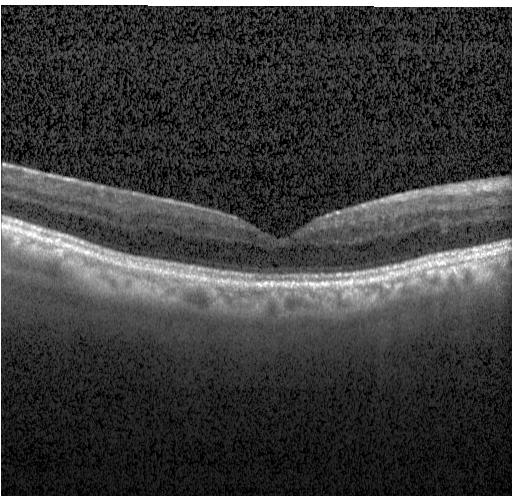

Retinal OCT cross-section. Heidelberg Spectralis OCT system. Spectral-domain OCT. Fovea-centered
Impression: no choroidal neovascularization, no diabetic macular edema, and no drusen.